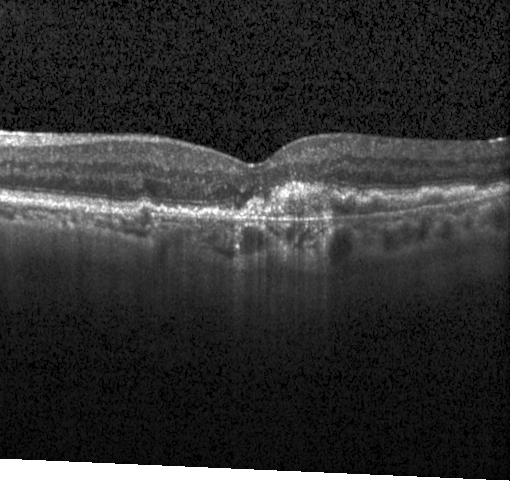

OCT B-scan; instrument: Heidelberg Spectralis; centered on the fovea
Finding: CNV.